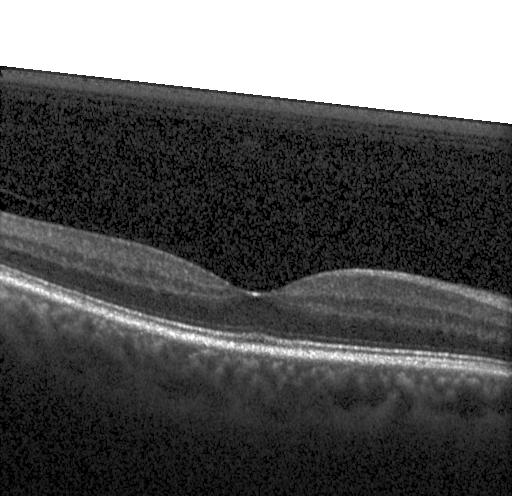

OCT line scan · macular scan — Dx: no CNV, no DME, and no drusen.